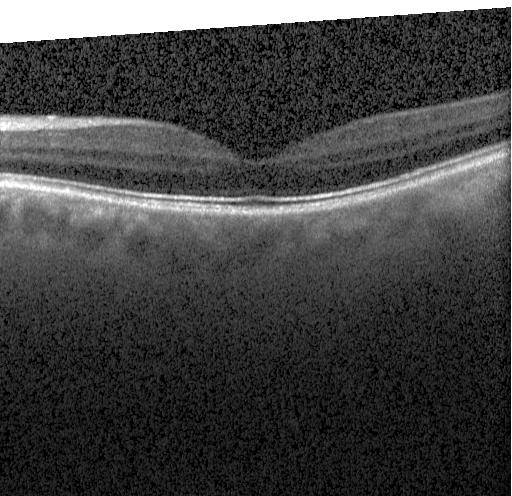 No choroidal neovascularization, diabetic macular edema, or drusen.